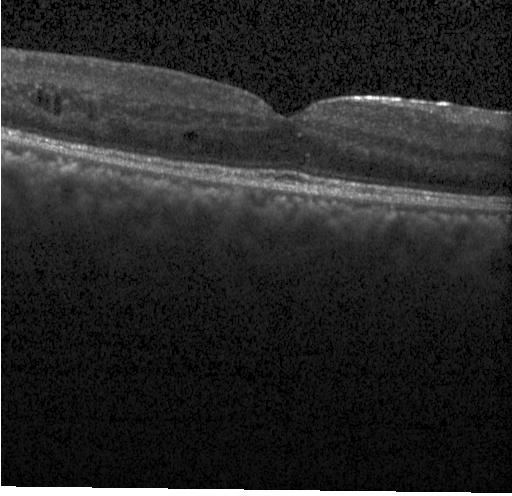 Horizontal scan through the fovea; optical coherence tomography scan; SD-OCT; Heidelberg Spectralis OCT system — Diagnosis: diabetic macular edema.